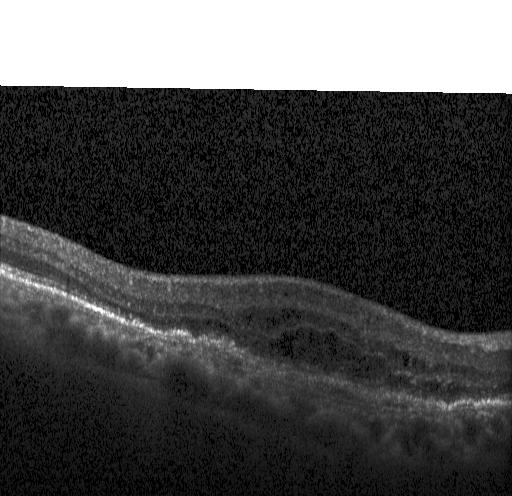 Fovea-centered; optical coherence tomography B-scan — Dx: a choroidal neovascular membrane.